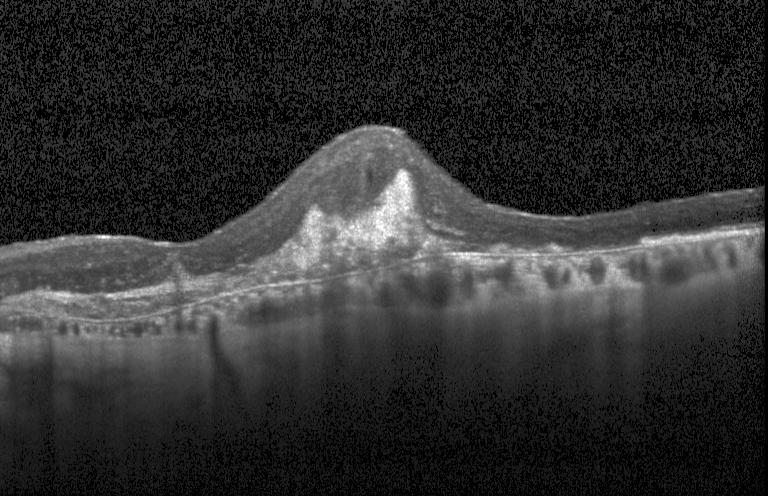

Instrument: Heidelberg Spectralis; retinal OCT cross-section — Dx: a choroidal neovascular membrane.